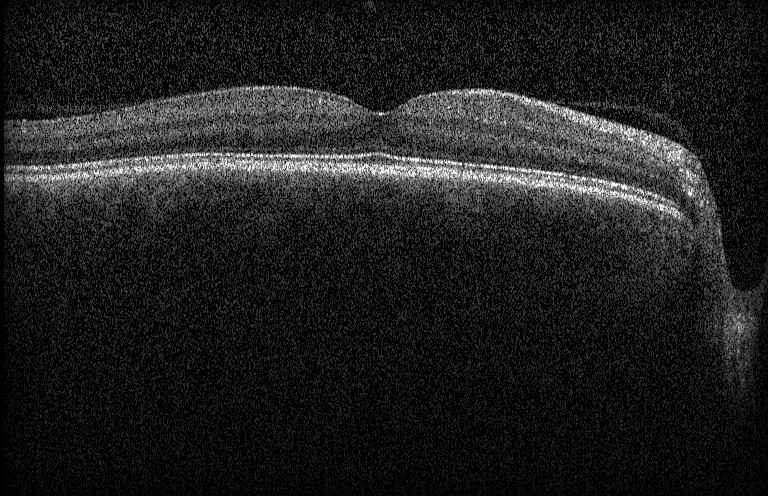

Fovea-centered; OCT line scan. No choroidal neovascularization, diabetic macular edema, or drusen.